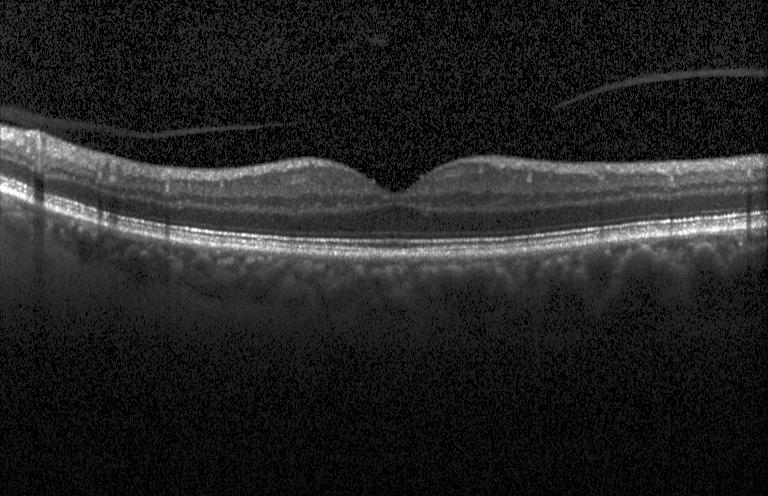
Retinal OCT cross-section showing no choroidal neovascularization, no diabetic macular edema, and no drusen.